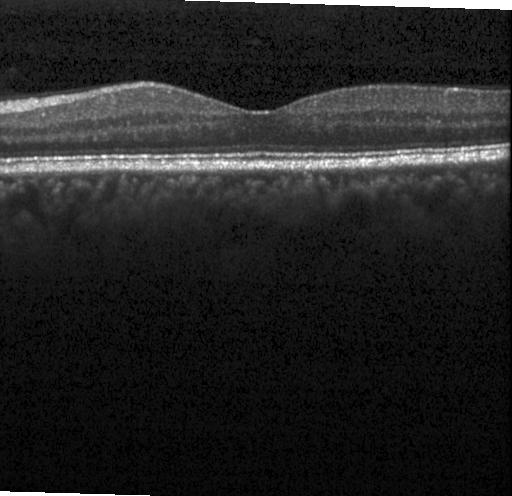

OCT B-scan.
Diagnosis: no CNV, no DME, and no drusen.